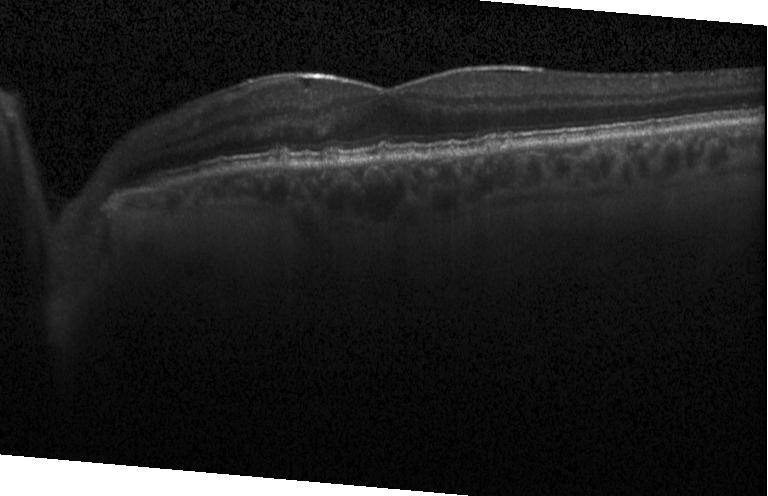

OCT scan showing multiple drusen.